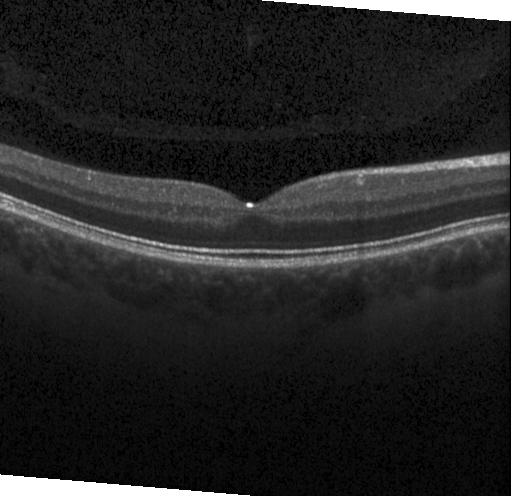

OCT finding: no evidence of choroidal neovascularization, diabetic macular edema, or drusen.